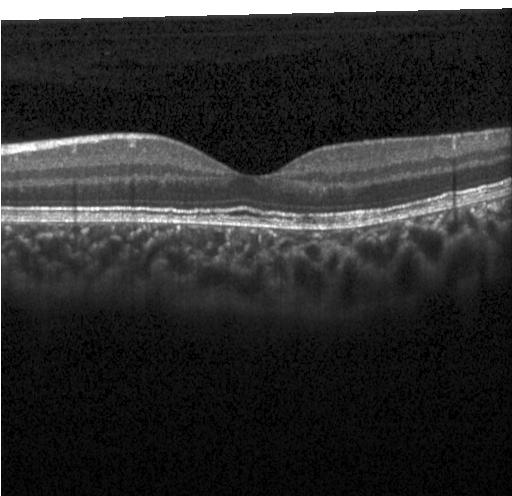

Macular OCT: no evidence of CNV, DME, or drusen.